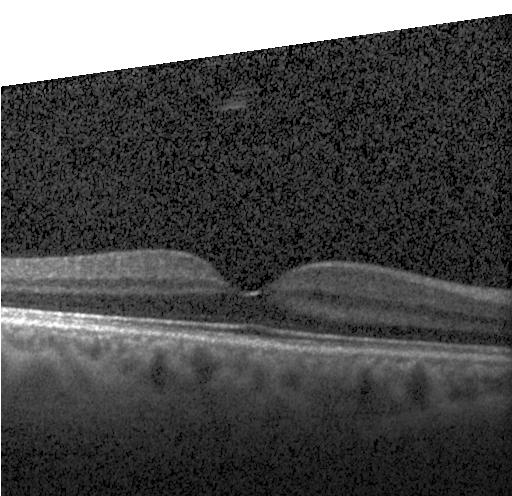
OCT line scan, horizontal scan through the fovea. Impression: no evidence of choroidal neovascularization, diabetic macular edema, or drusen.